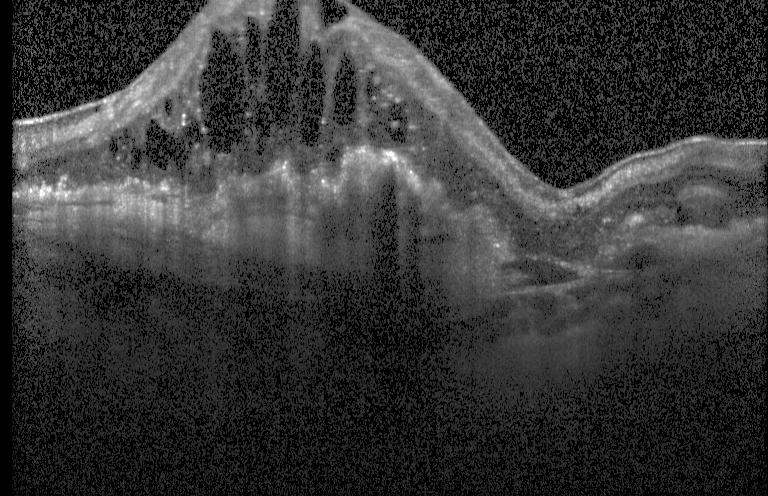 Heidelberg Spectralis OCT system. OCT line scan. Finding: CNV.